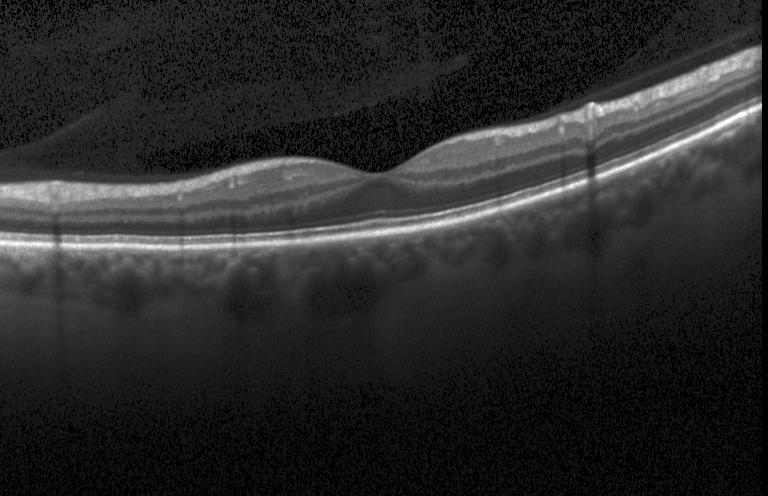 Heidelberg Spectralis OCT system; retinal OCT B-scan; spectral-domain optical coherence tomography.
Dx: no choroidal neovascularization, no diabetic macular edema, and no drusen.